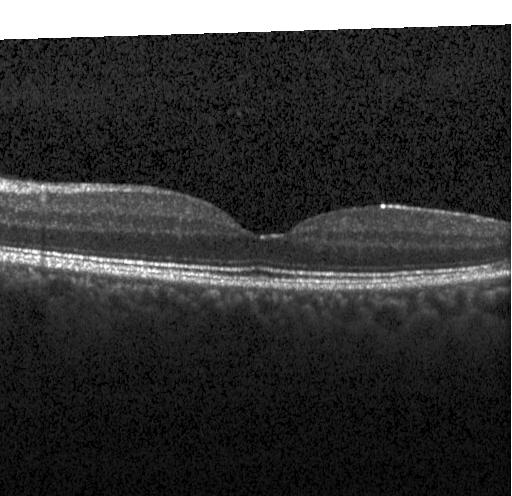

SD-OCT, Heidelberg Spectralis OCT system, fovea-centered, retinal OCT cross-section
Diagnosis: no evidence of choroidal neovascularization, diabetic macular edema, or drusen.